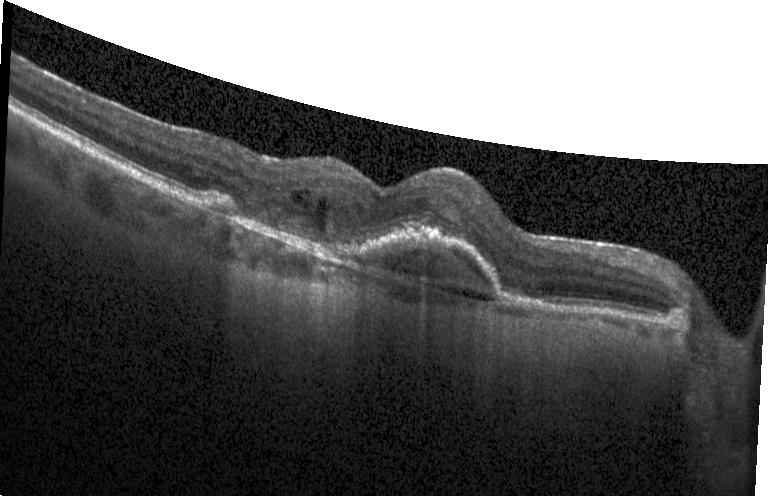 Impression: choroidal neovascularization.